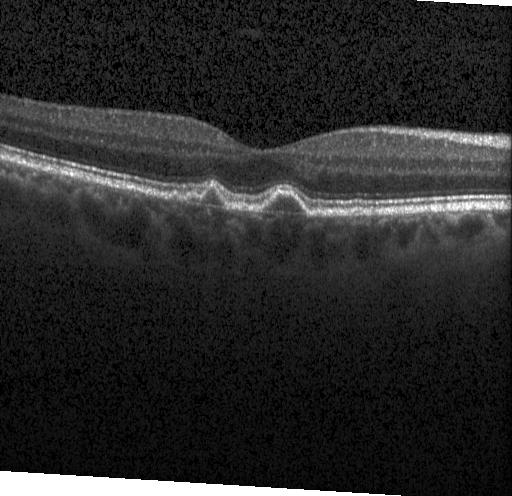

Spectral-domain OCT. Centered on the fovea. OCT B-scan. Finding: sub-RPE drusenoid deposits.